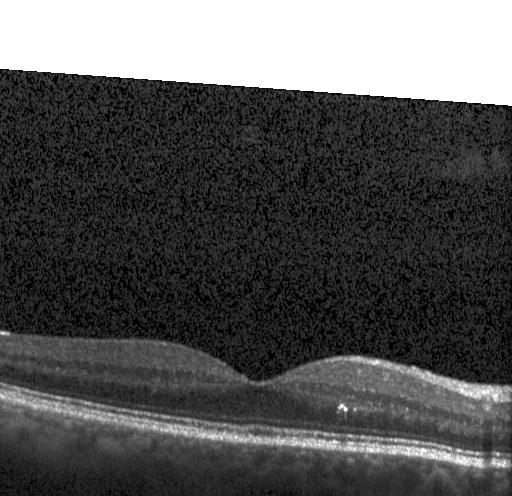 Through the macula · spectral-domain optical coherence tomography · optical coherence tomography scan · Heidelberg Spectralis OCT system.
Impression: no CNV, DME, or drusen.